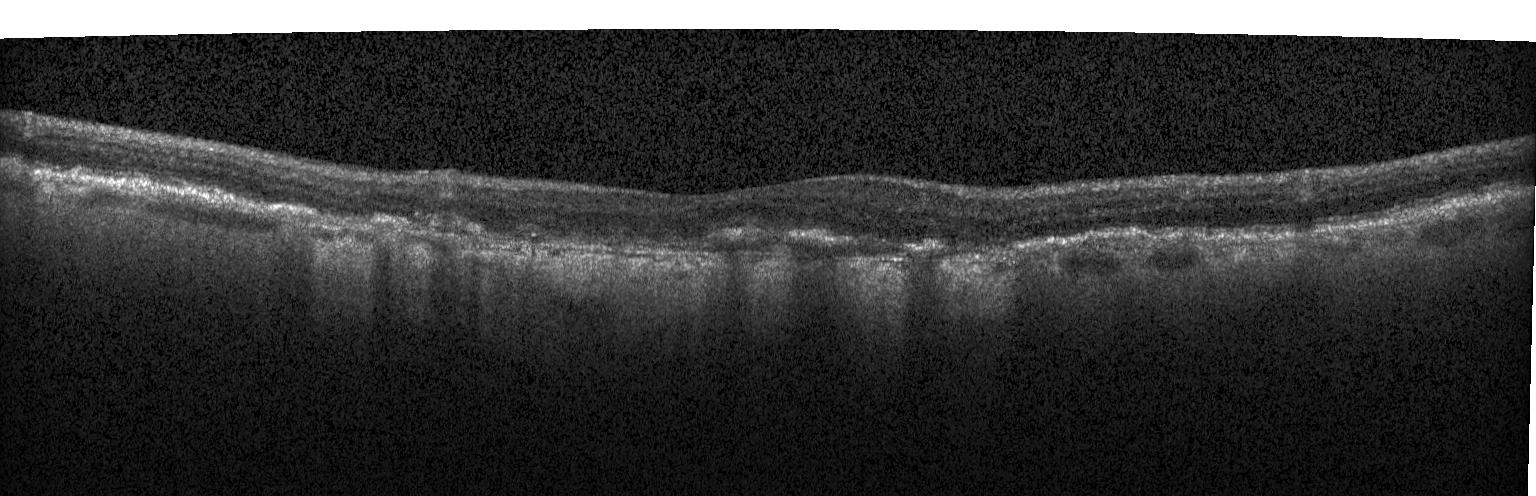

Horizontal scan through the fovea, instrument: Heidelberg Spectralis, retinal OCT cross-section.
Impression: a choroidal neovascular membrane.